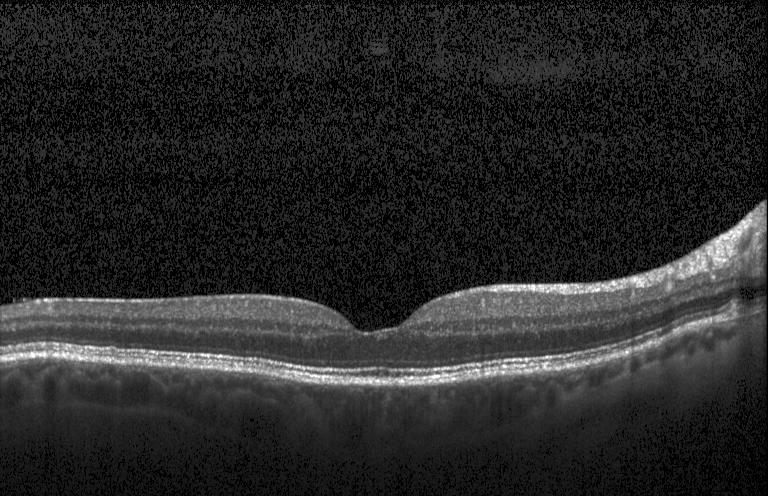

OCT line scan; centered on the fovea; acquired on a Heidelberg Spectralis — Assessment: no choroidal neovascularization, diabetic macular edema, or drusen.